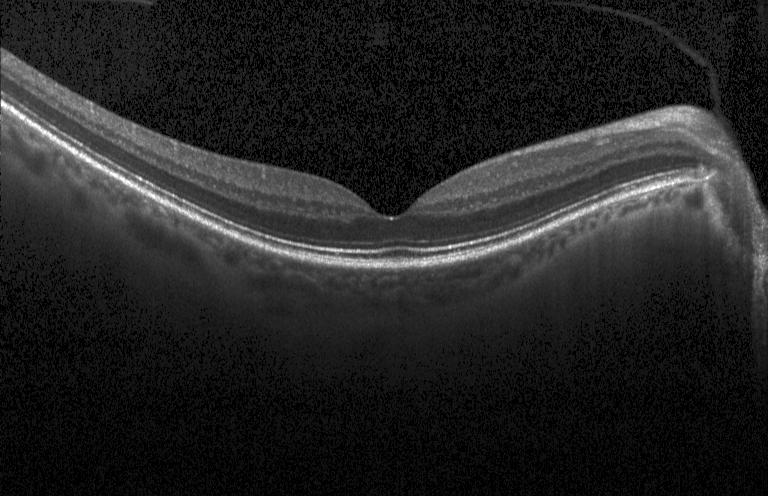
OCT scan showing no evidence of choroidal neovascularization, diabetic macular edema, or drusen.